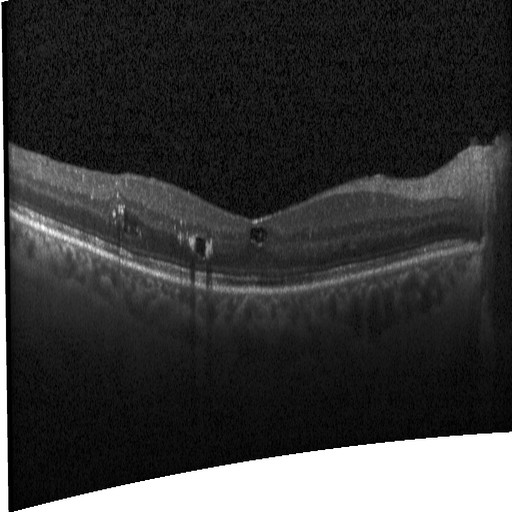
Spectral-domain OCT · Heidelberg Spectralis · retinal OCT cross-section · through the macula. Diabetic macular edema (DME).